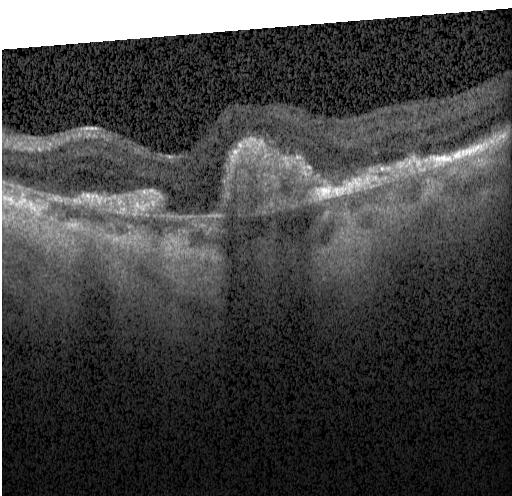

Heidelberg Spectralis. Retinal OCT B-scan. Horizontal scan through the fovea. Spectral-domain OCT — Dx: a choroidal neovascular membrane.